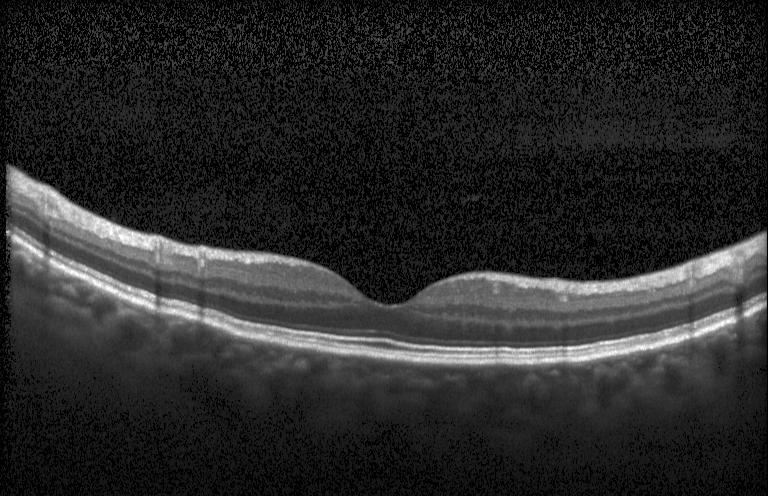 Spectral-domain OCT · fovea-centered · optical coherence tomography scan
Diagnosis: no evidence of choroidal neovascularization, diabetic macular edema, or drusen.